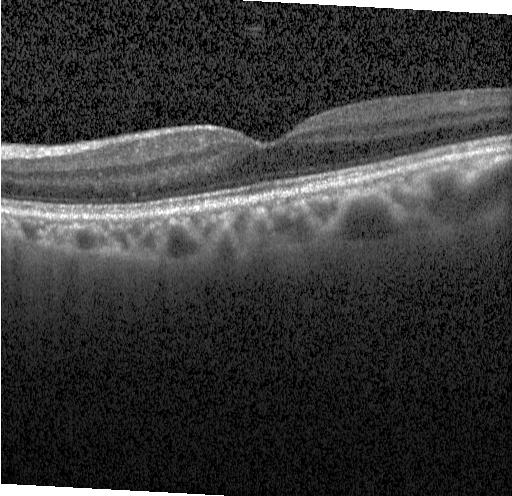
Optical coherence tomography B-scan.
The scan shows no CNV, DME, or drusen.